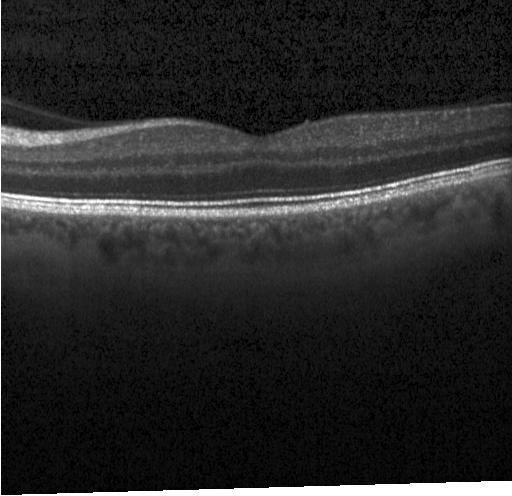
OCT scan showing no evidence of choroidal neovascularization, diabetic macular edema, or drusen.